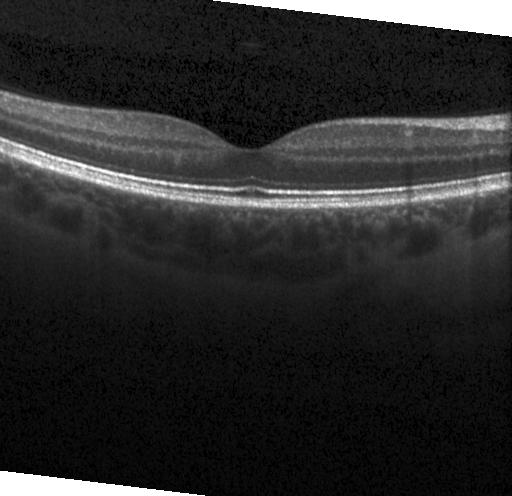 Optical coherence tomography scan — Finding: neither choroidal neovascularization, diabetic macular edema, nor drusen.